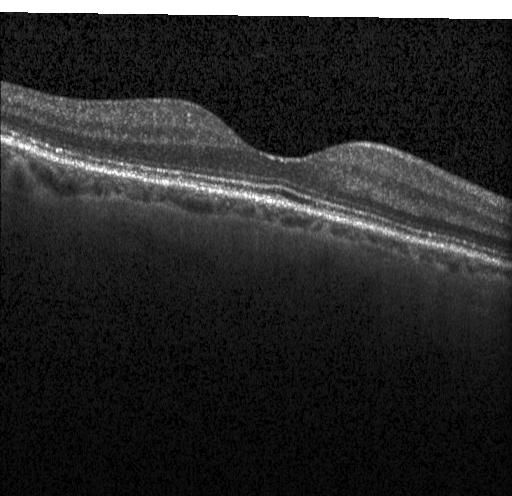 Instrument: Heidelberg Spectralis, retinal OCT cross-section. This B-scan demonstrates no CNV, DME, or drusen.